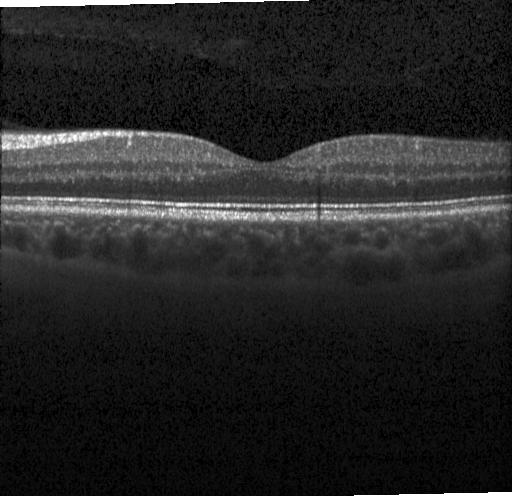
Retinal OCT cross-section
Diagnosis: neither choroidal neovascularization, diabetic macular edema, nor drusen.